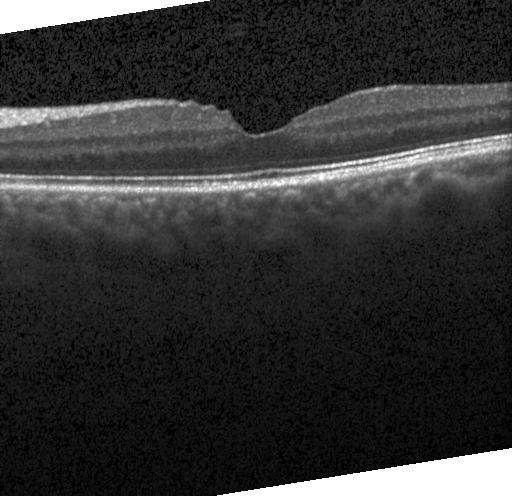
Diagnosis: no choroidal neovascularization, diabetic macular edema, or drusen.